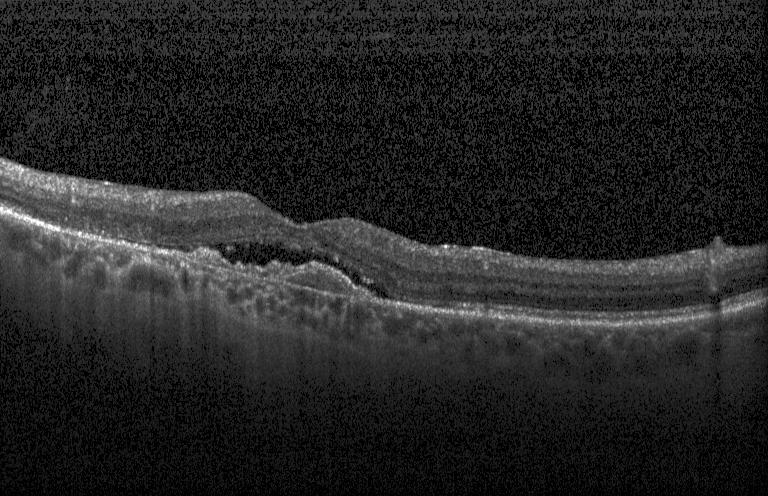
Retinal OCT B-scan.
Macular OCT: choroidal neovascularization.